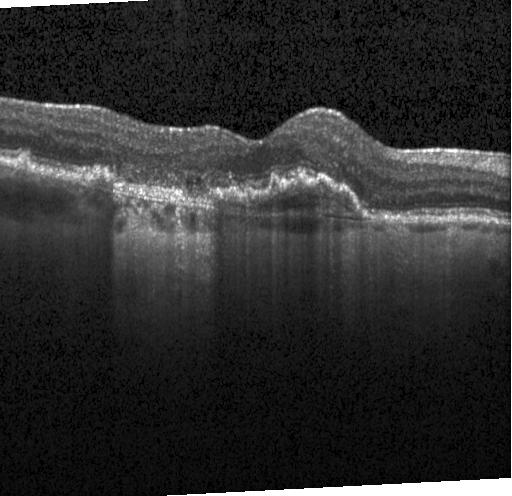

SD-OCT · OCT B-scan — Finding: a choroidal neovascular membrane.